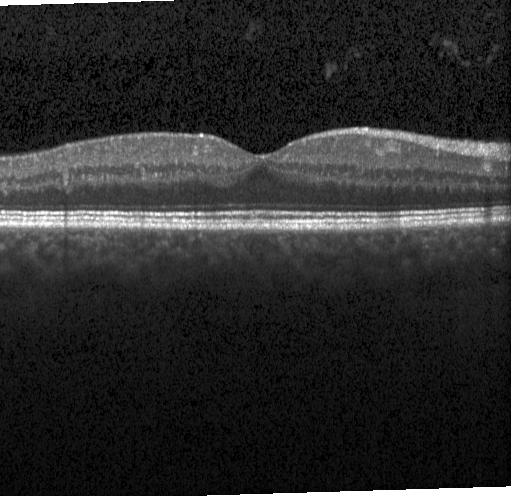 Optical coherence tomography B-scan · Heidelberg Spectralis · SD-OCT — Finding: no CNV, DME, or drusen.